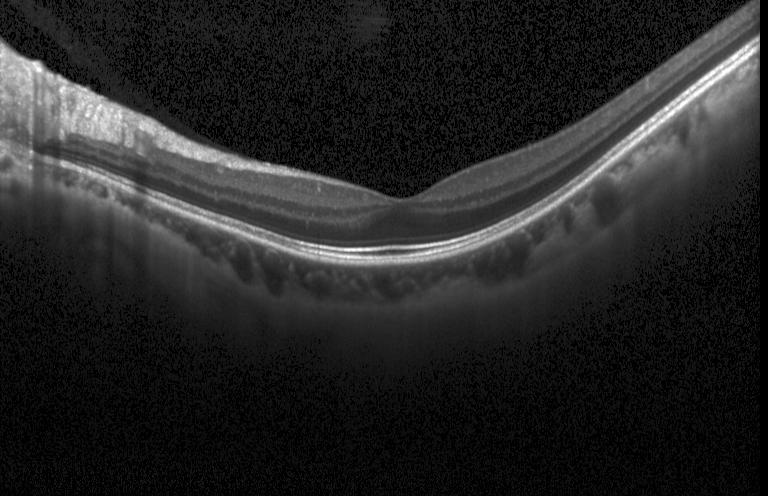 Spectral-domain OCT. Through the macula. Retinal OCT B-scan.
Dx: neither CNV, DME, nor drusen.